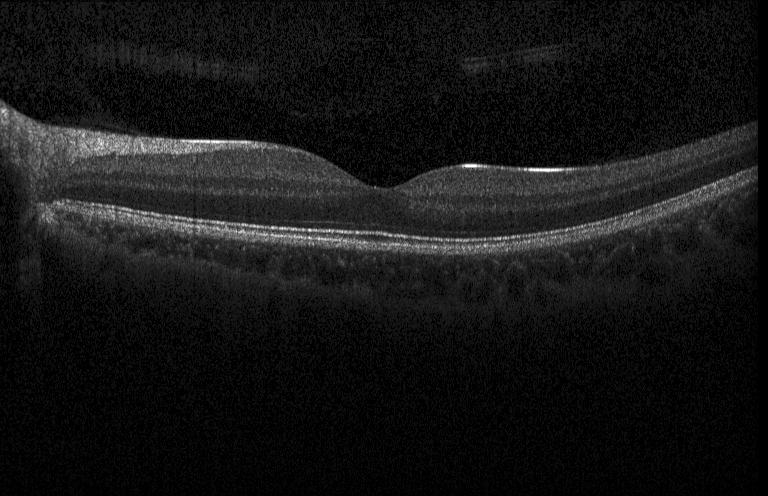

Spectral-domain optical coherence tomography · optical coherence tomography scan · Heidelberg Spectralis OCT system
Diagnosis: no choroidal neovascularization, diabetic macular edema, or drusen.